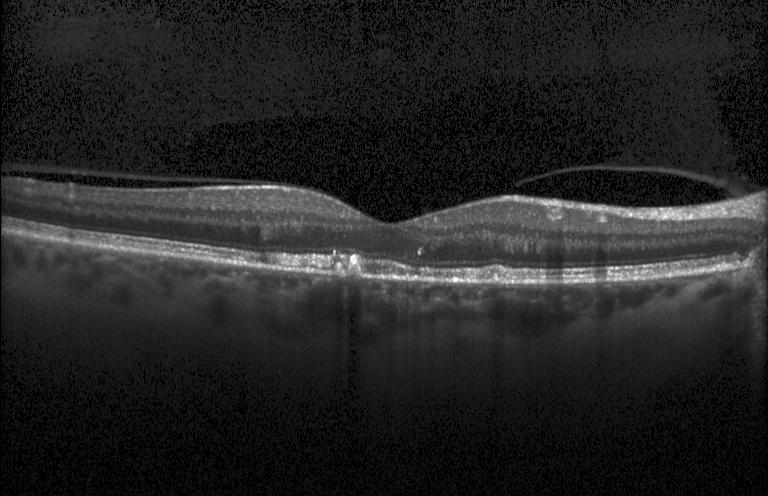

Dx: sub-RPE drusenoid deposits.